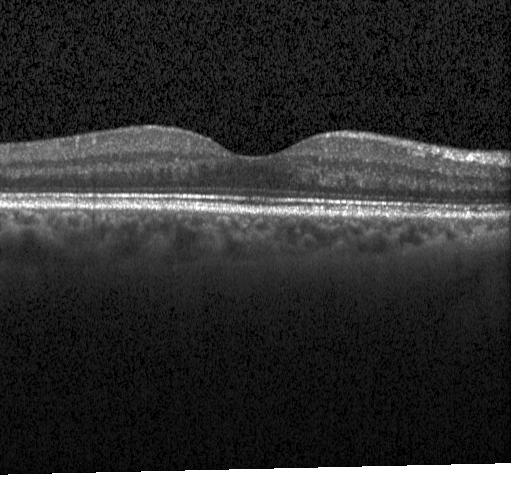
Horizontal scan through the fovea, OCT B-scan. OCT finding: no CNV, no DME, and no drusen.